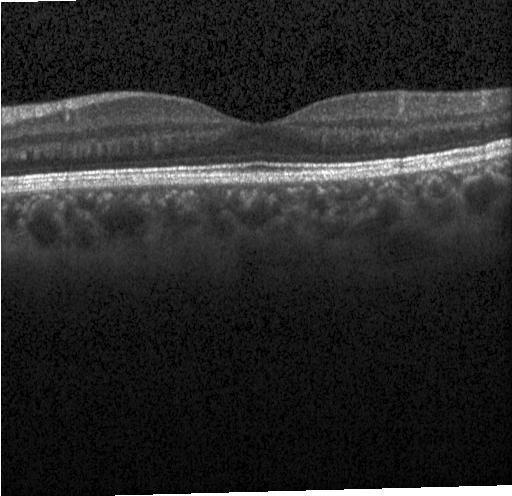

Optical coherence tomography B-scan.
Impression: no choroidal neovascularization, diabetic macular edema, or drusen.